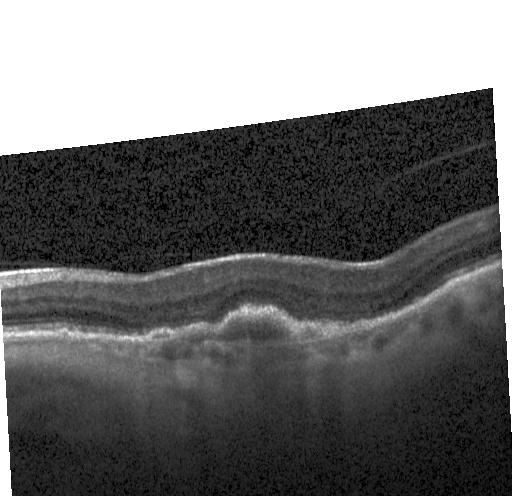
Dx: a choroidal neovascular membrane.